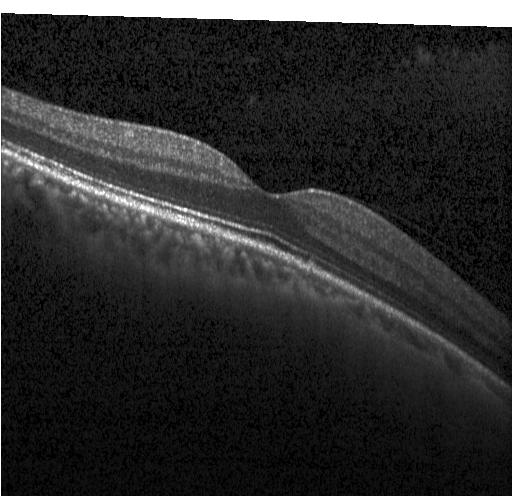

Retinal OCT cross-section showing neither choroidal neovascularization, diabetic macular edema, nor drusen.